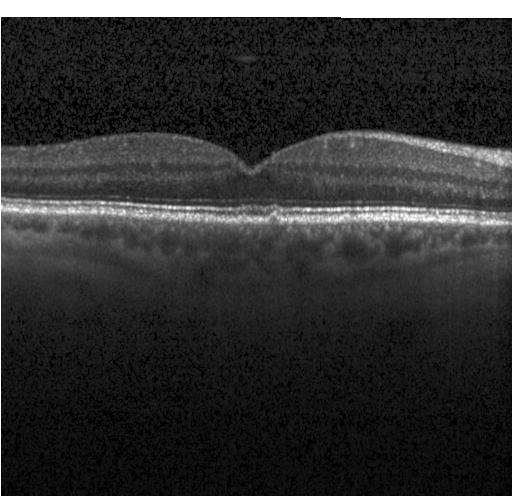

Impression: sub-RPE drusenoid deposits.